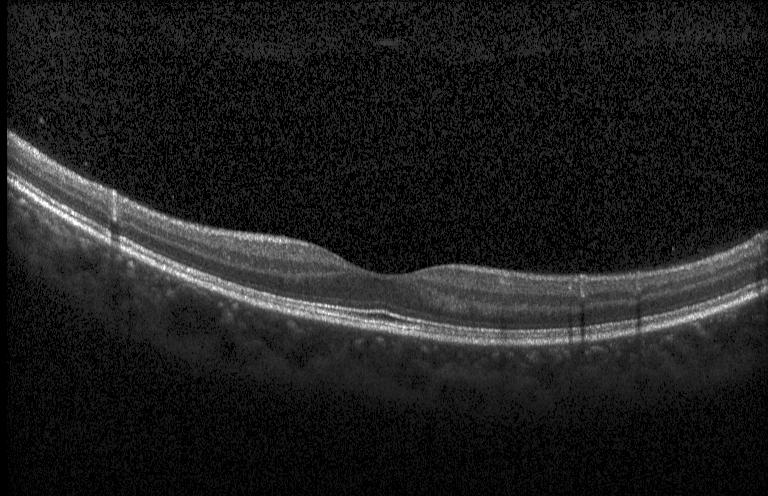 This B-scan demonstrates no evidence of choroidal neovascularization, diabetic macular edema, or drusen.